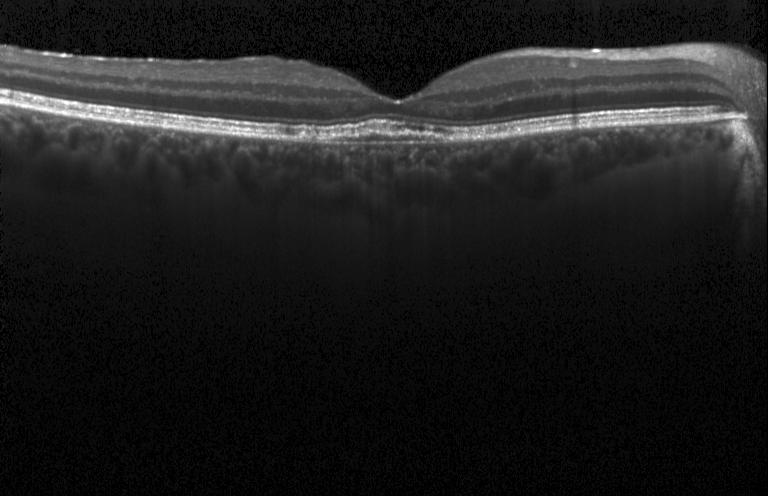

OCT B-scan; instrument: Heidelberg Spectralis; centered on the fovea
Finding: CNV.